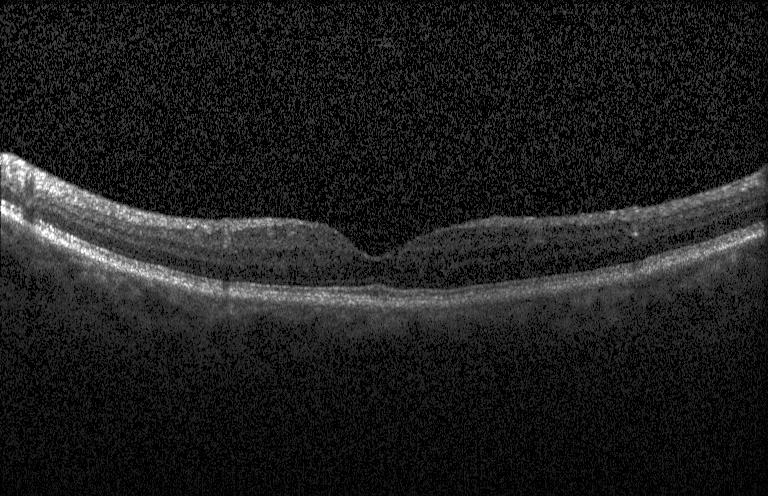 No evidence of CNV, DME, or drusen.